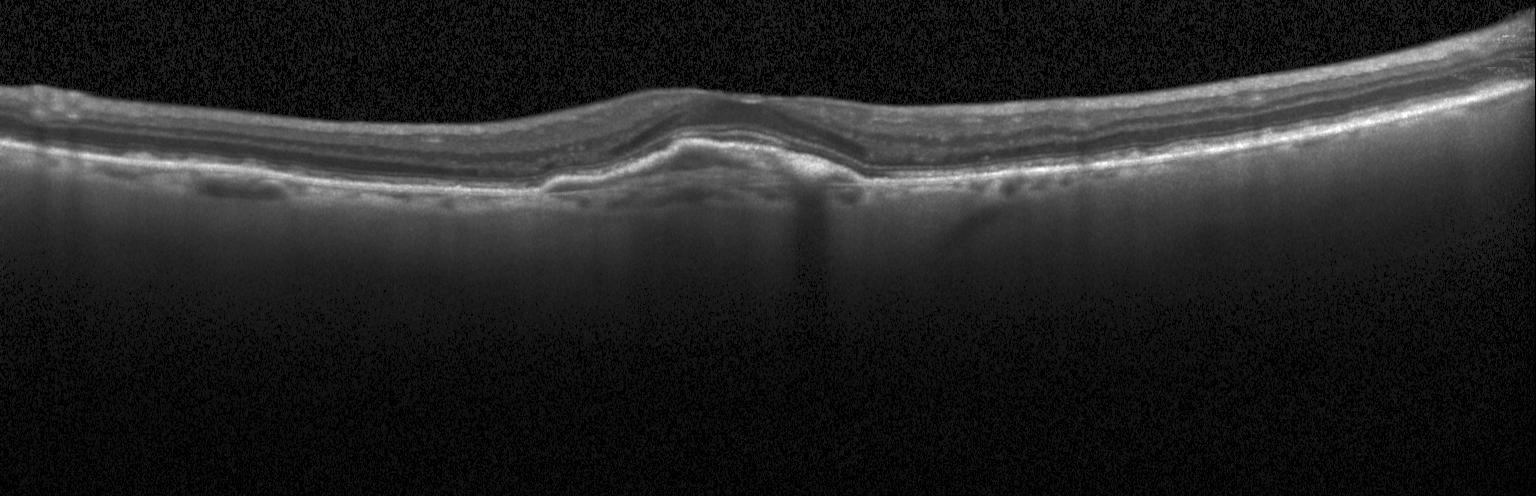

Impression: a choroidal neovascular membrane.